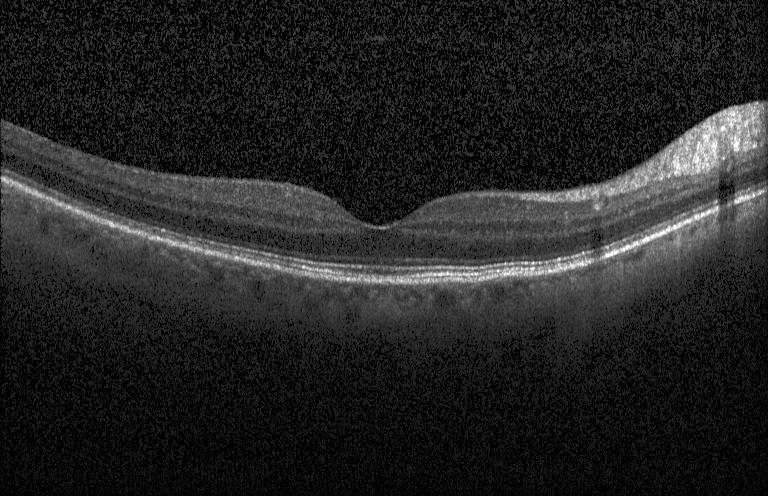
Spectral-domain OCT B-scan: no evidence of CNV, DME, or drusen.